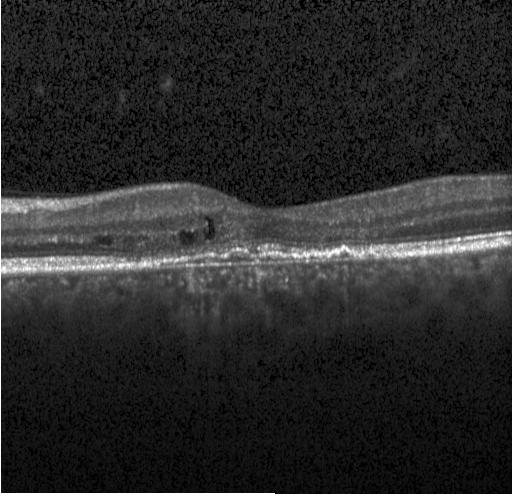
Optical coherence tomography scan; through the macula
A choroidal neovascular membrane.